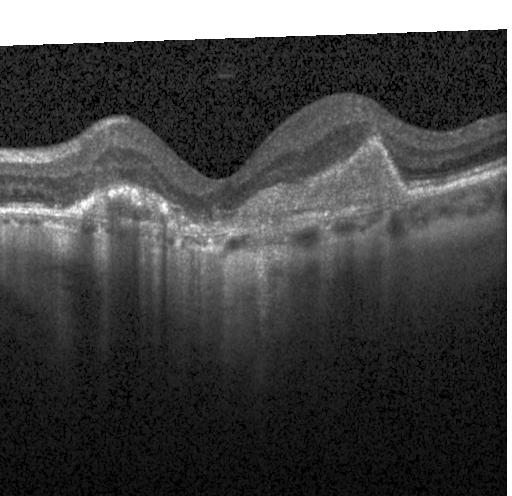
Heidelberg Spectralis. OCT line scan.
OCT finding: choroidal neovascularization (CNV).